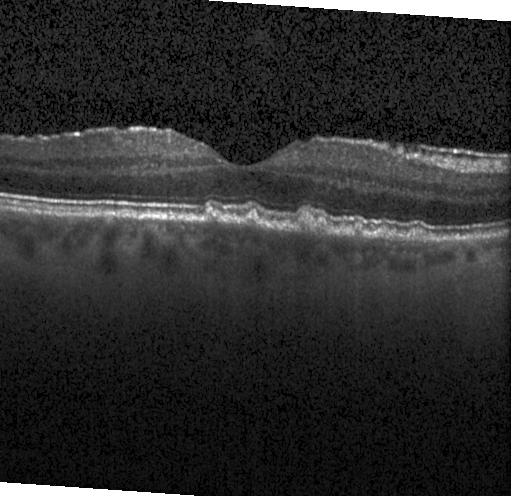 Fovea-centered; SD-OCT; retinal OCT B-scan. Finding: sub-RPE drusenoid deposits.